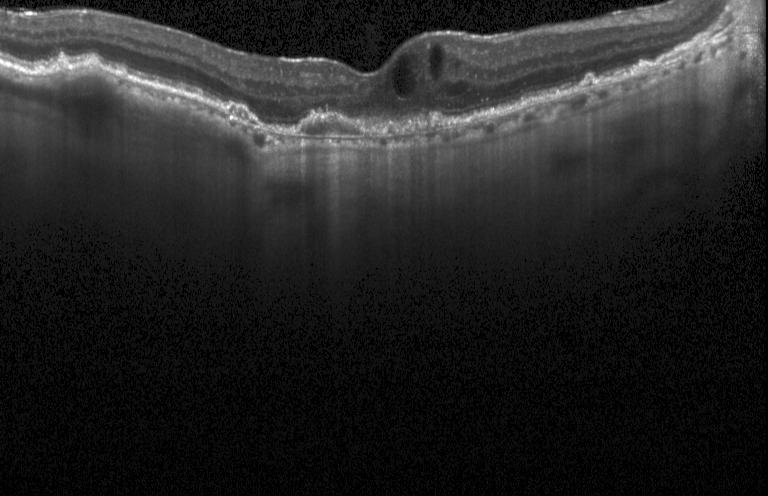 Retinal OCT cross-section
Finding: choroidal neovascularization.